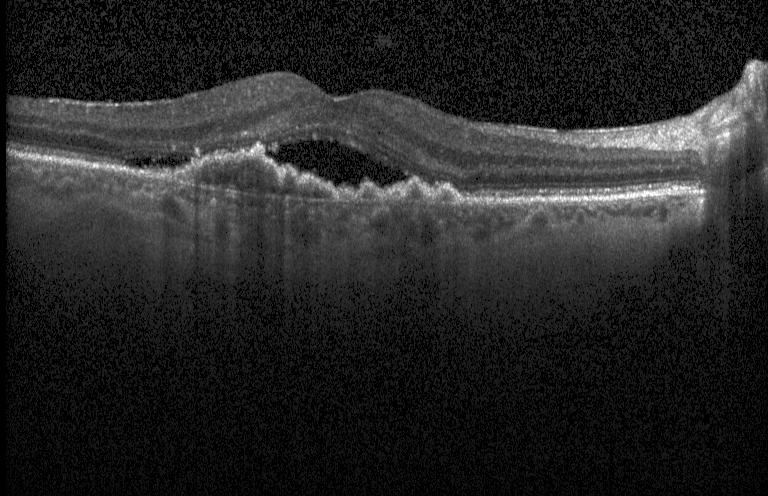

Heidelberg Spectralis · optical coherence tomography B-scan · spectral-domain optical coherence tomography — Finding: choroidal neovascularization (CNV).